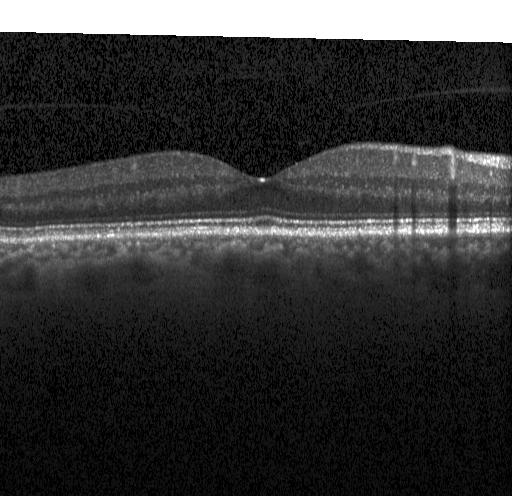

Horizontal scan through the fovea, optical coherence tomography scan.
Impression: no choroidal neovascularization, diabetic macular edema, or drusen.